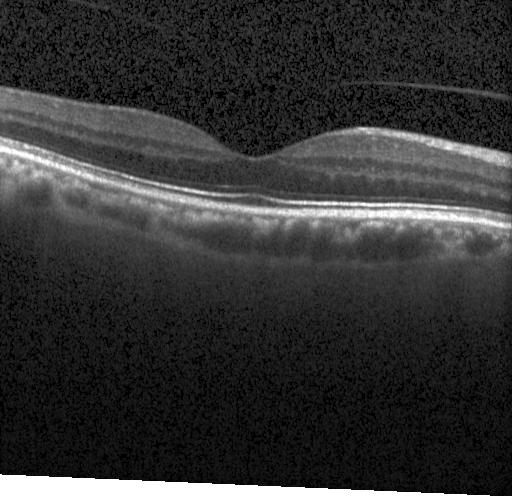

Retinal OCT cross-section. Spectral-domain optical coherence tomography. Heidelberg Spectralis — No choroidal neovascularization, diabetic macular edema, or drusen.